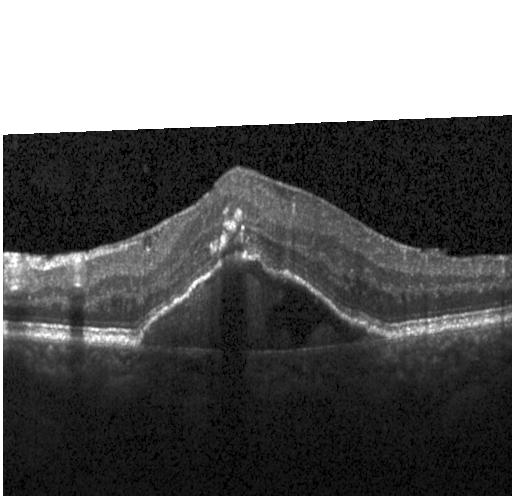

Optical coherence tomography B-scan. SD-OCT. Through the macula
Impression: a choroidal neovascular membrane.